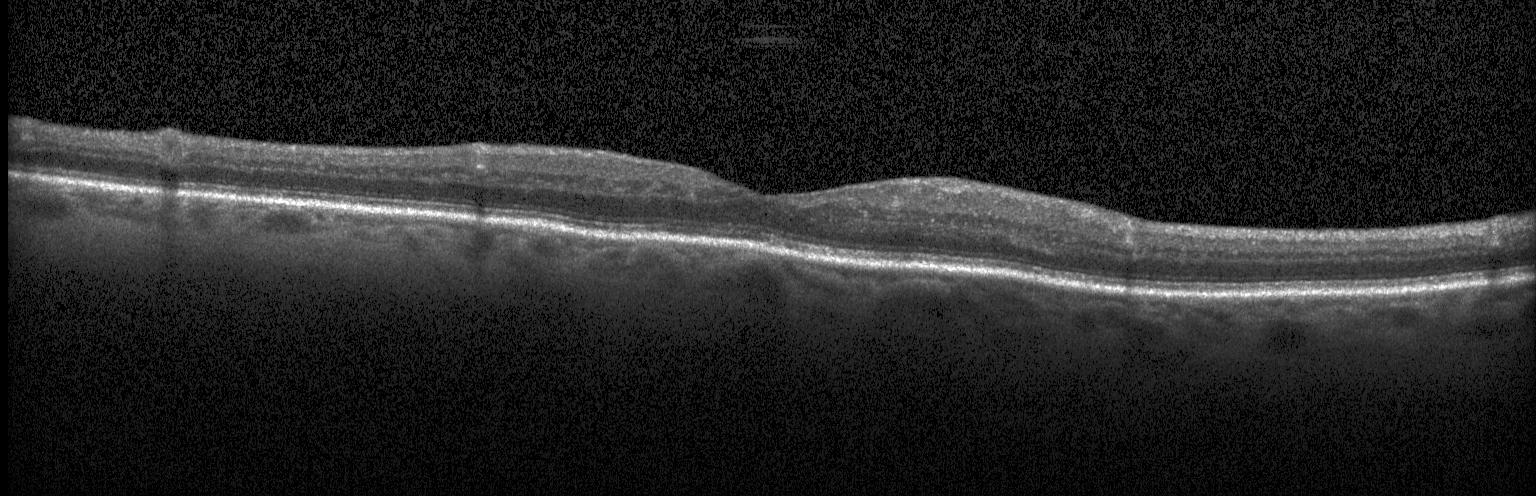
Spectral-domain OCT B-scan: no CNV, no DME, and no drusen.